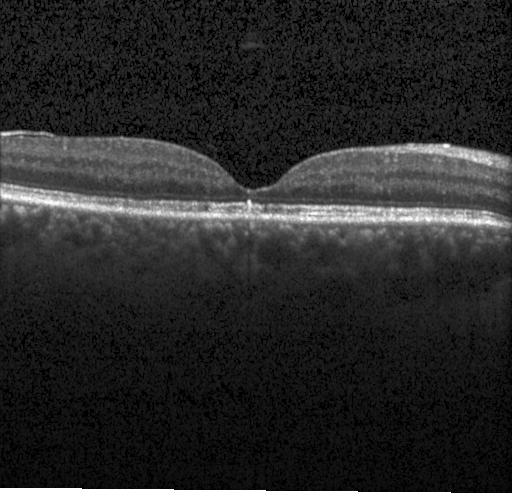 Diagnosis: neither choroidal neovascularization, diabetic macular edema, nor drusen.